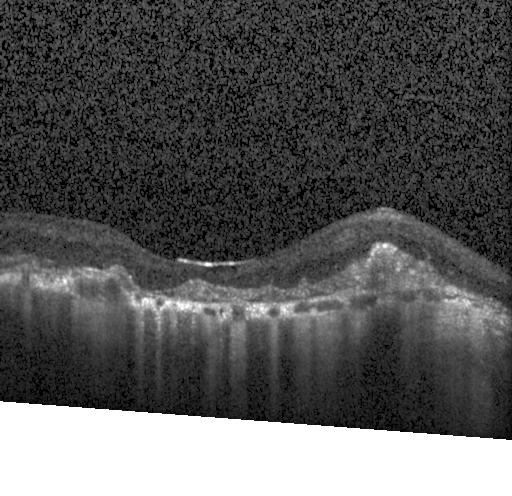
Instrument: Heidelberg Spectralis. Retinal OCT cross-section. Diagnosis: choroidal neovascularization (CNV).